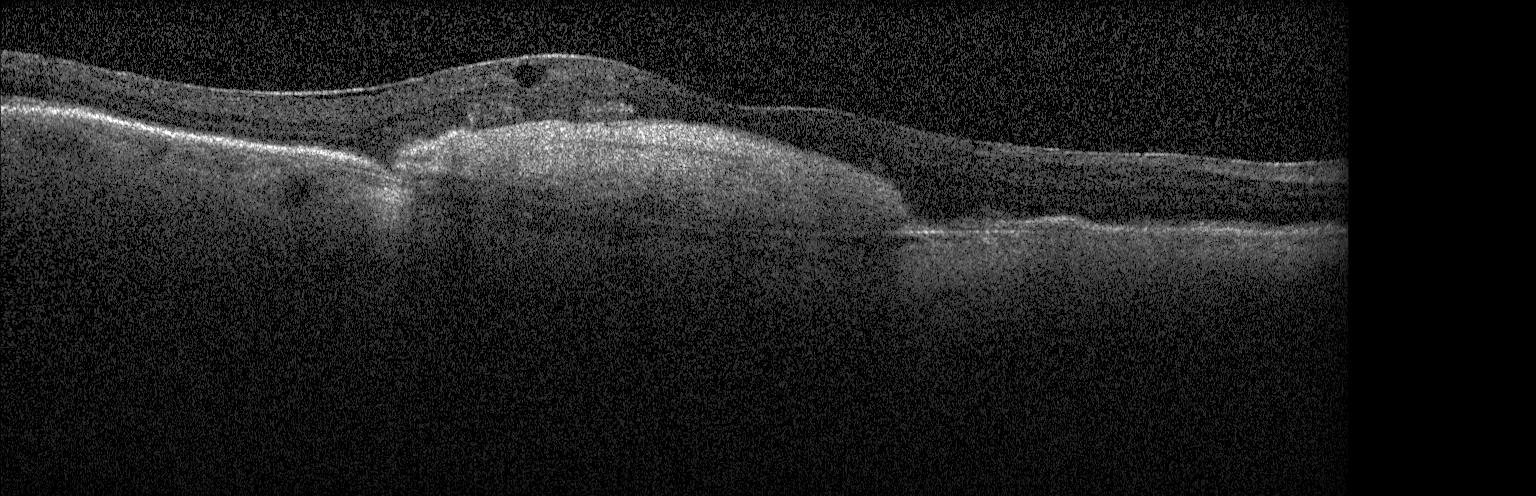

OCT line scan. Fovea-centered. SD-OCT. Acquired on a Heidelberg Spectralis.
Diagnosis: CNV.